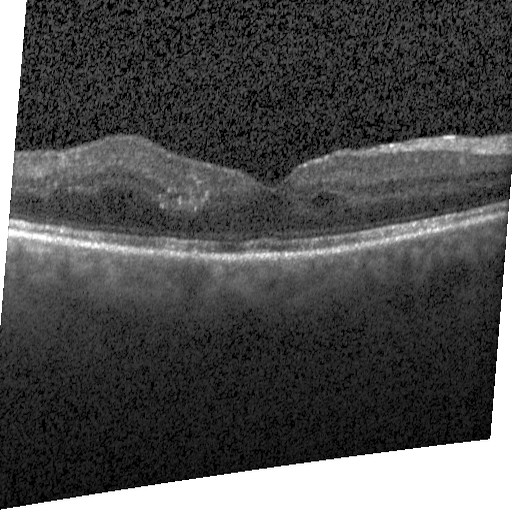 OCT finding: diabetic macular edema (DME).